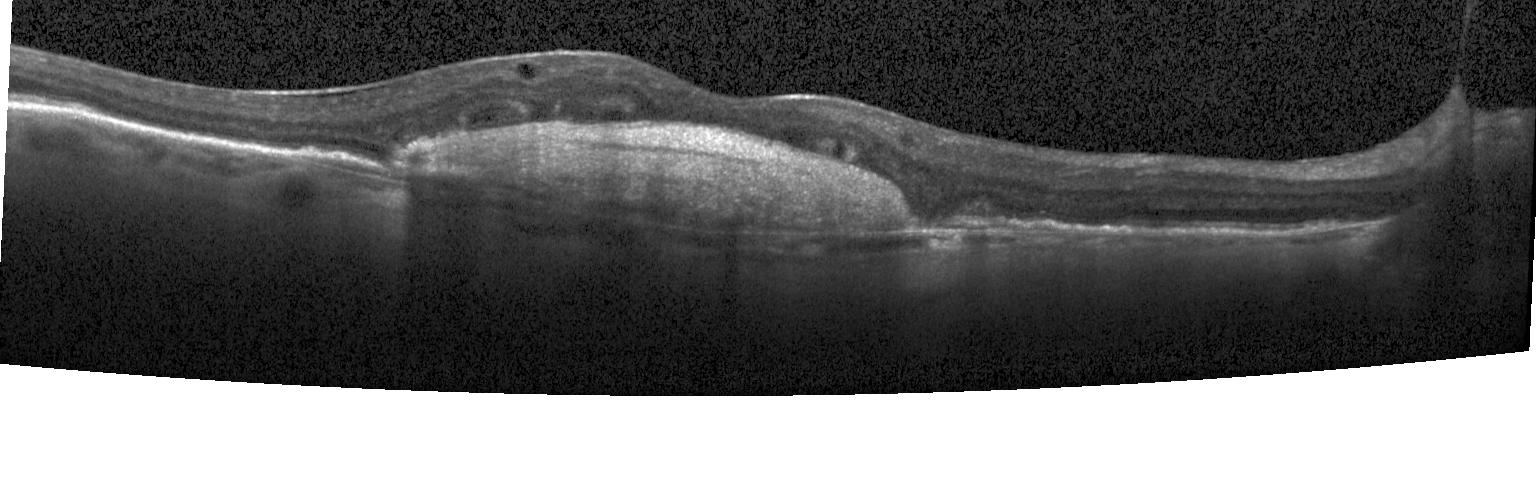

Optical coherence tomography B-scan · acquired on a Heidelberg Spectralis
The scan shows choroidal neovascularization.